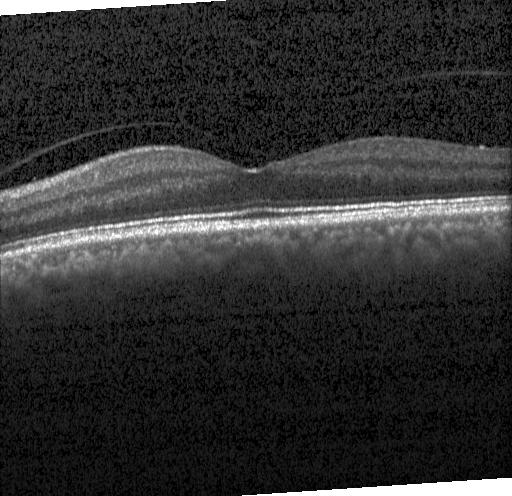

Finding: neither choroidal neovascularization, diabetic macular edema, nor drusen.